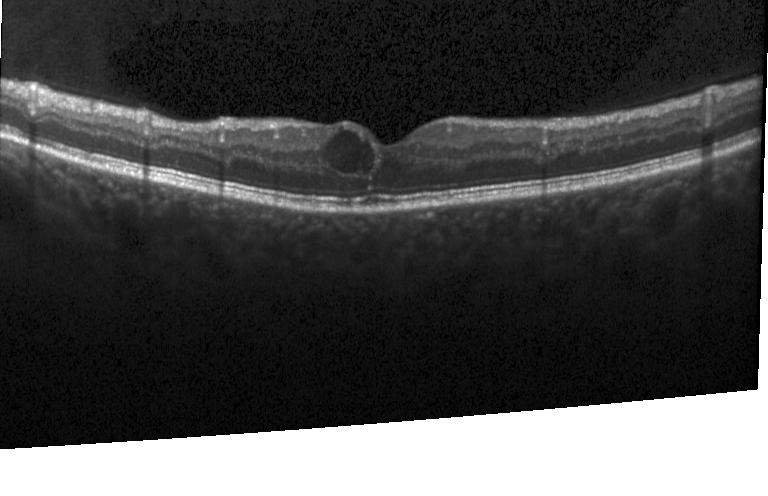
Heidelberg Spectralis, fovea-centered, spectral-domain optical coherence tomography, optical coherence tomography scan
OCT finding: diabetic macular edema.